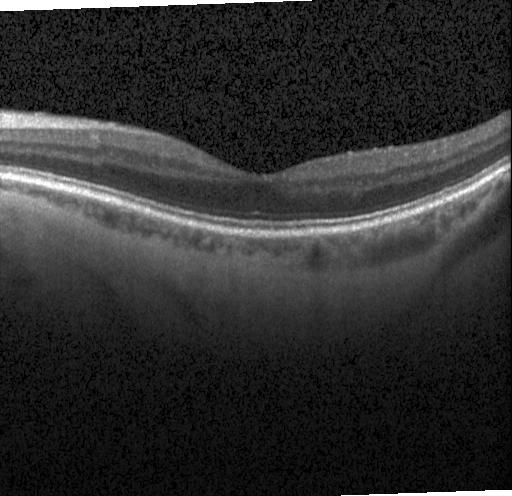
Retinal OCT B-scan — The scan shows no evidence of choroidal neovascularization, diabetic macular edema, or drusen.